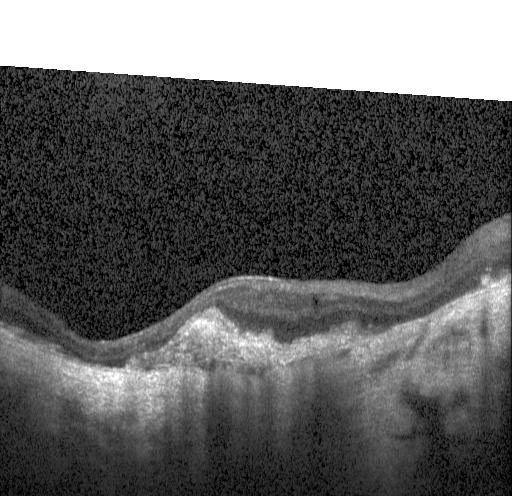 Retinal OCT cross-section, centered on the fovea, spectral-domain OCT. Finding: a choroidal neovascular membrane.